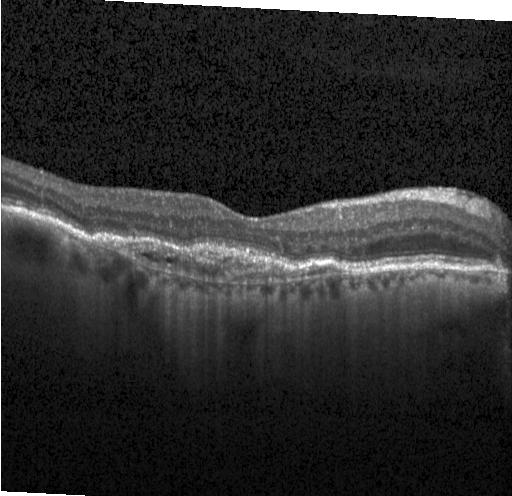
Finding: CNV.